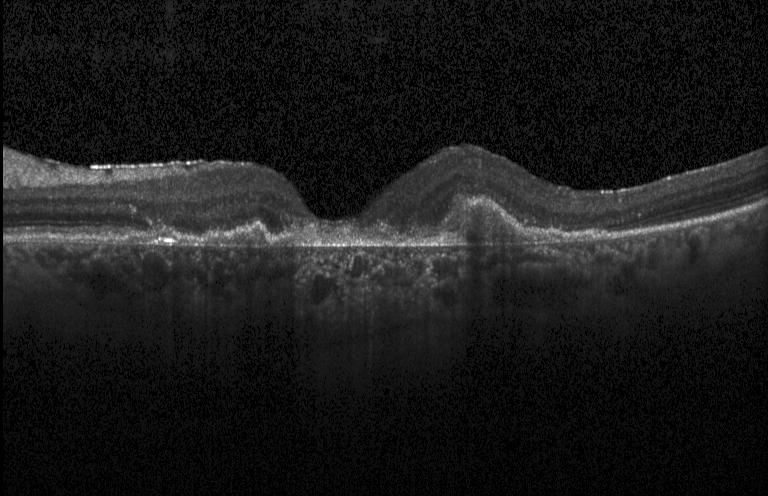
Macular scan. SD-OCT. OCT line scan. Acquired on a Heidelberg Spectralis. The scan shows a choroidal neovascular membrane.